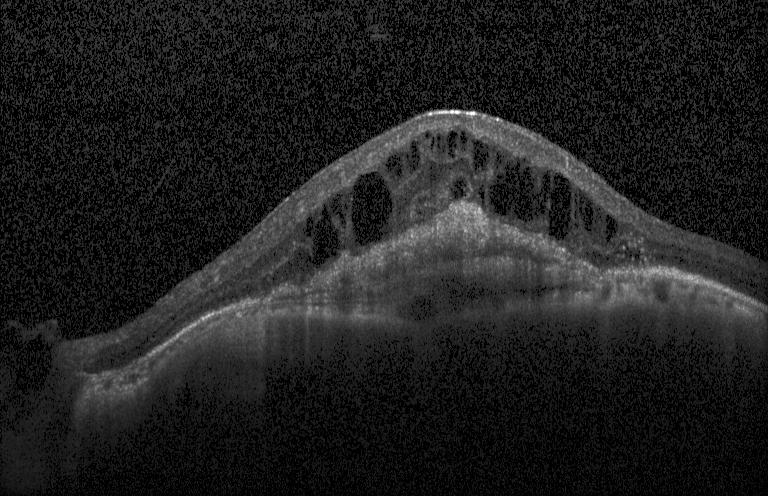
OCT B-scan.
A choroidal neovascular membrane.